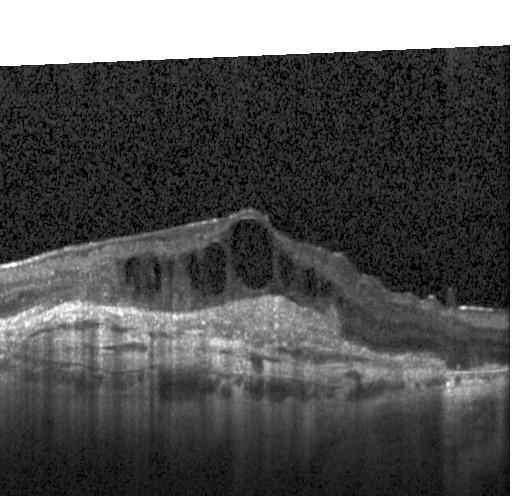
Optical coherence tomography scan · instrument: Heidelberg Spectralis · fovea-centered · spectral-domain optical coherence tomography
The scan shows a choroidal neovascular membrane.